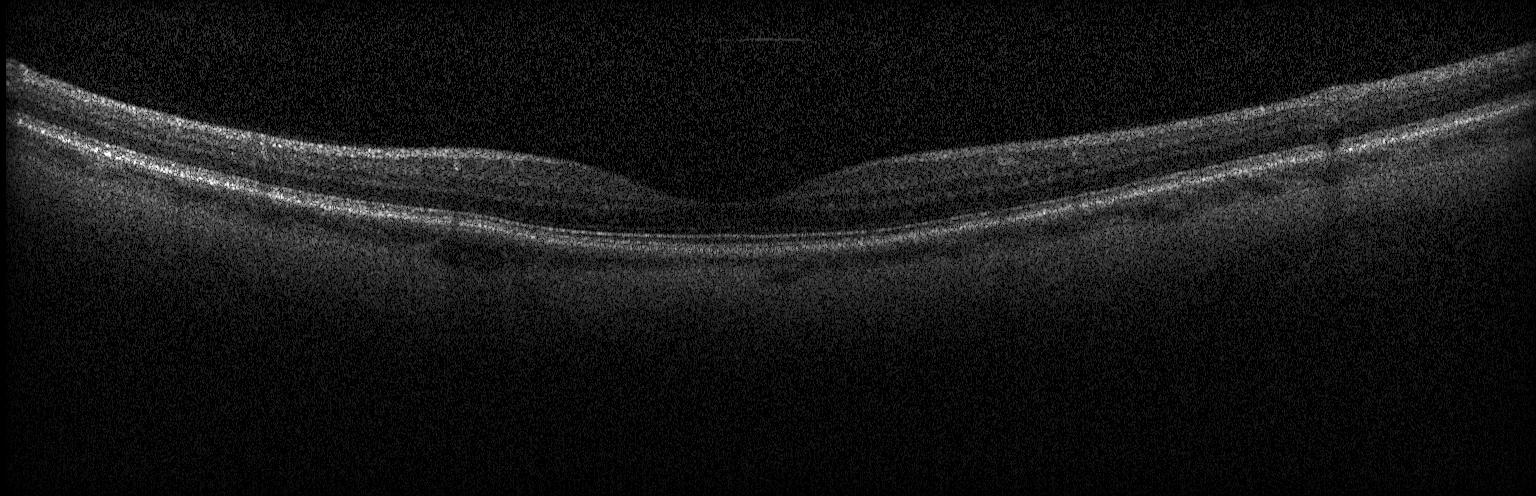
Retinal OCT cross-section — Diagnosis: no evidence of choroidal neovascularization, diabetic macular edema, or drusen.